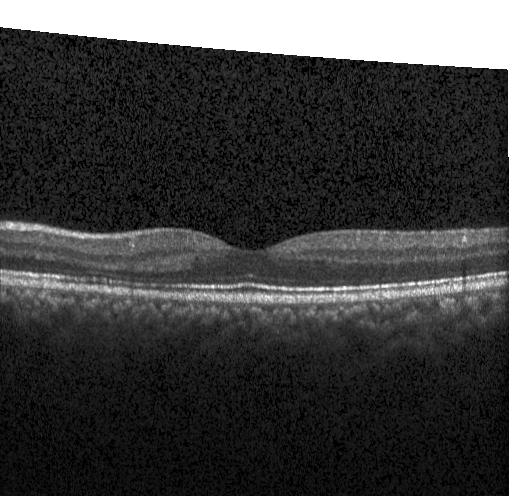

OCT B-scan.
Finding: no choroidal neovascularization, diabetic macular edema, or drusen.